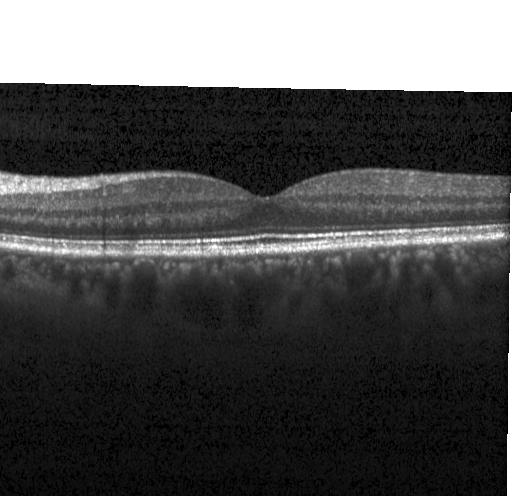
Retinal OCT cross-section showing no CNV, DME, or drusen.